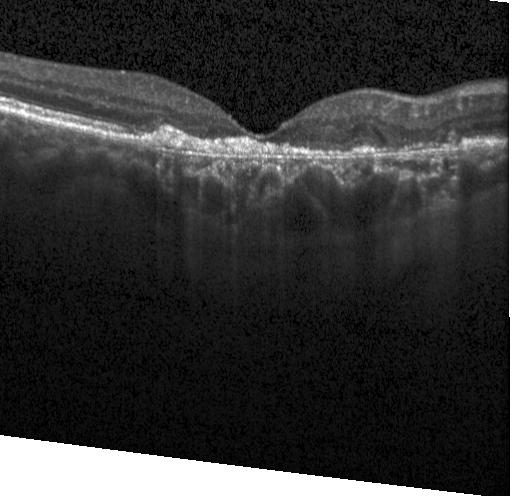
Dx: choroidal neovascularization (CNV).